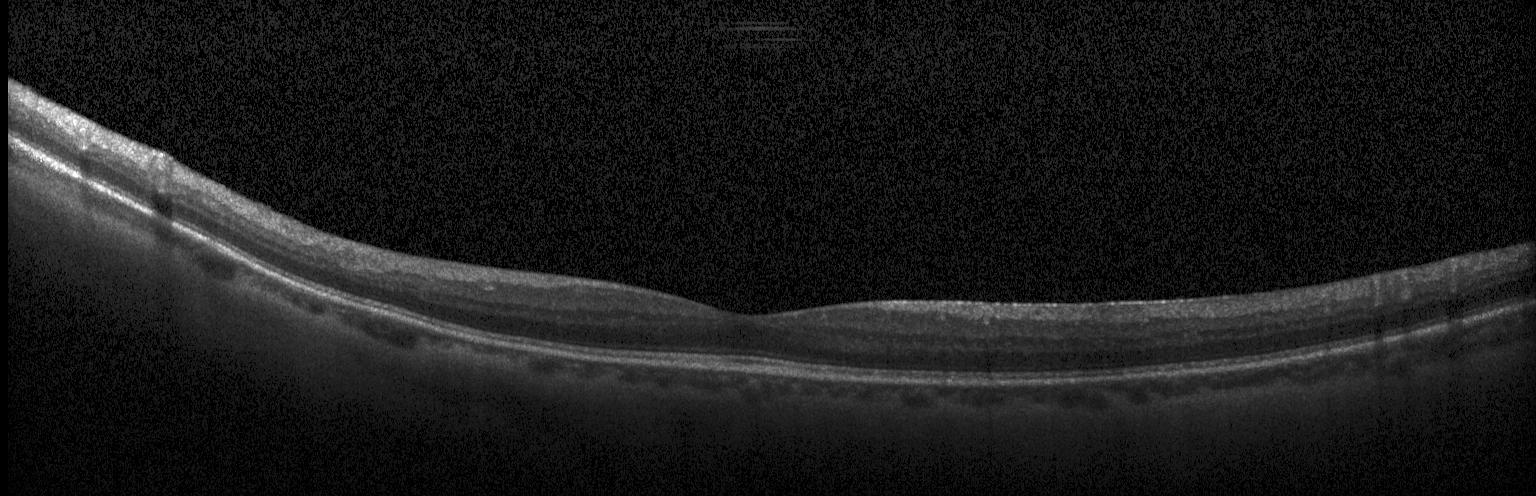
Retinal OCT B-scan — Assessment: neither choroidal neovascularization, diabetic macular edema, nor drusen.